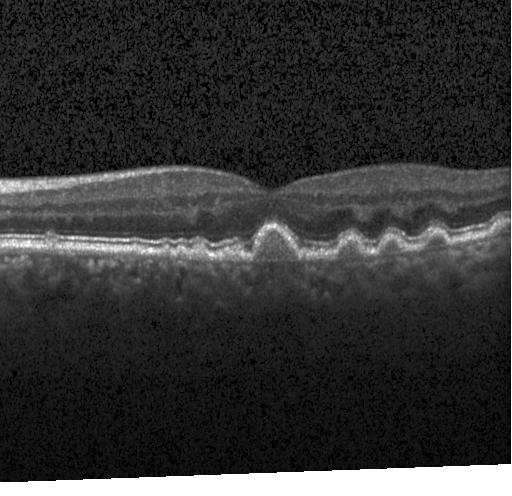 OCT finding: sub-RPE drusenoid deposits.